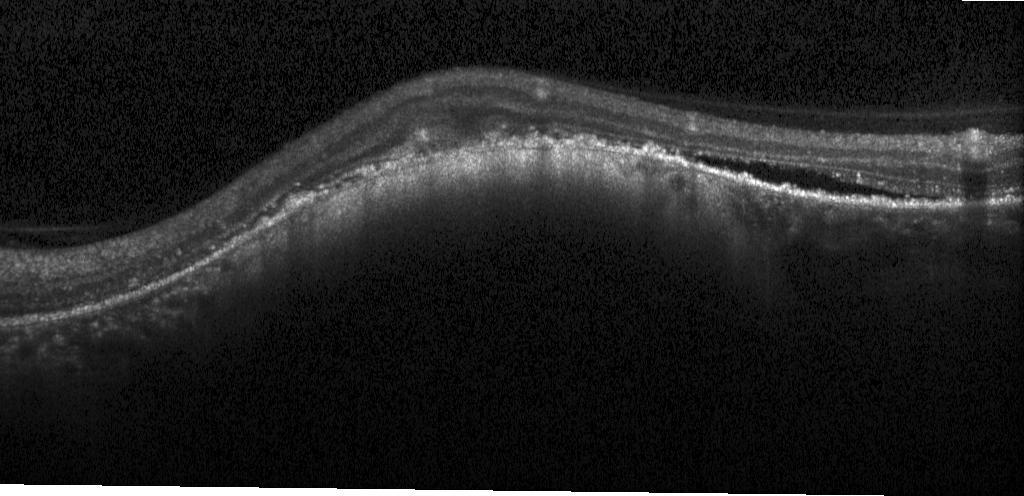

Macular OCT demonstrating choroidal neovascularization.